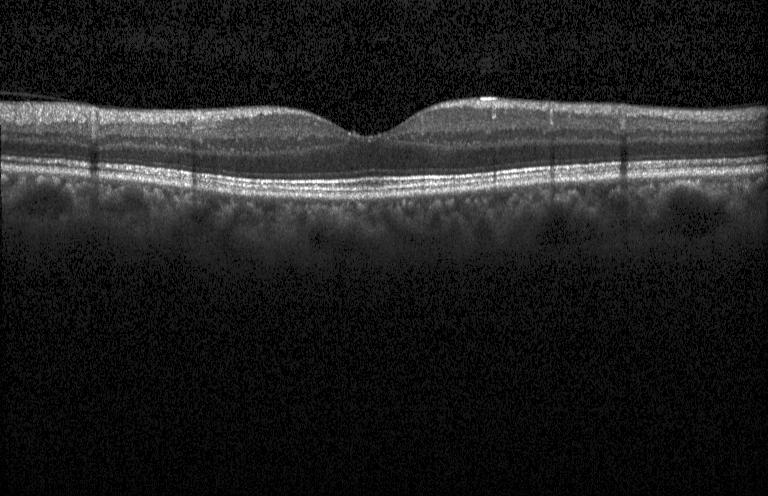

No choroidal neovascularization, no diabetic macular edema, and no drusen.